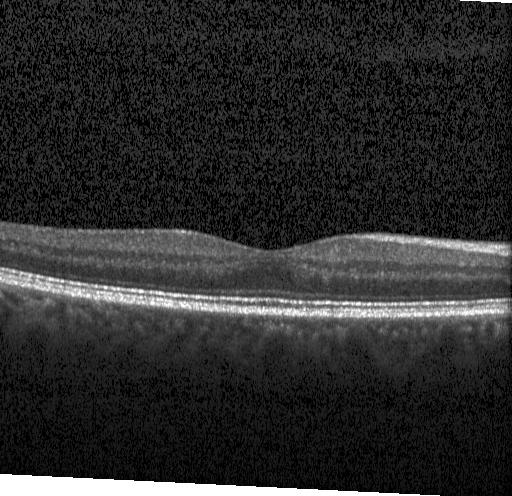 Through the macula · retinal OCT B-scan · Heidelberg Spectralis · spectral-domain OCT
Diagnosis: neither choroidal neovascularization, diabetic macular edema, nor drusen.